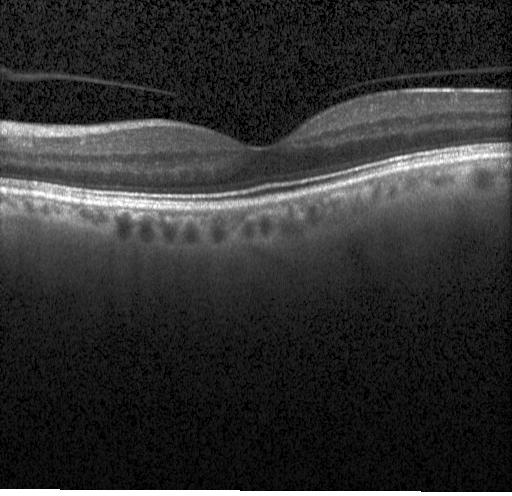
Retinal OCT cross-section — This B-scan demonstrates no evidence of CNV, DME, or drusen.